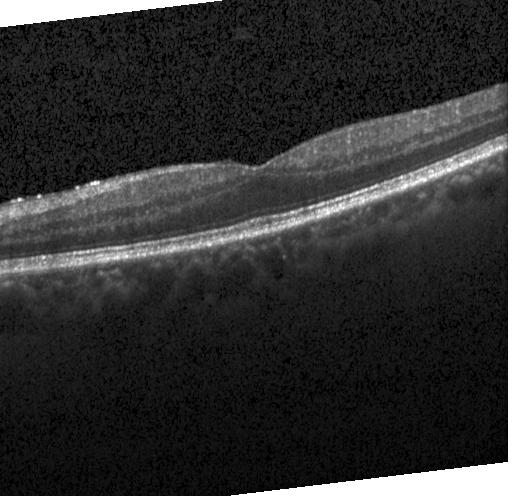
Horizontal scan through the fovea · optical coherence tomography scan
Finding: no CNV, no DME, and no drusen.